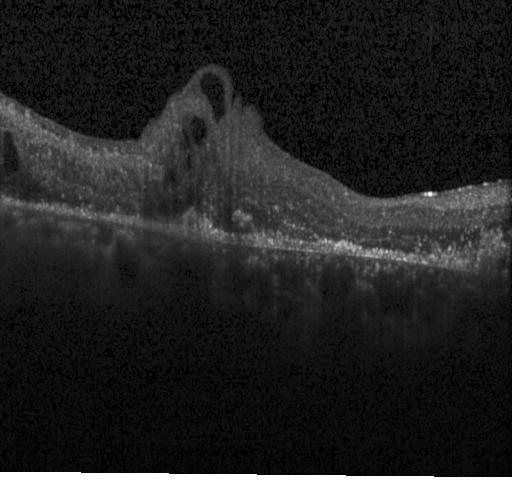

Heidelberg Spectralis OCT system, retinal OCT cross-section, spectral-domain optical coherence tomography
Diagnosis: a choroidal neovascular membrane.